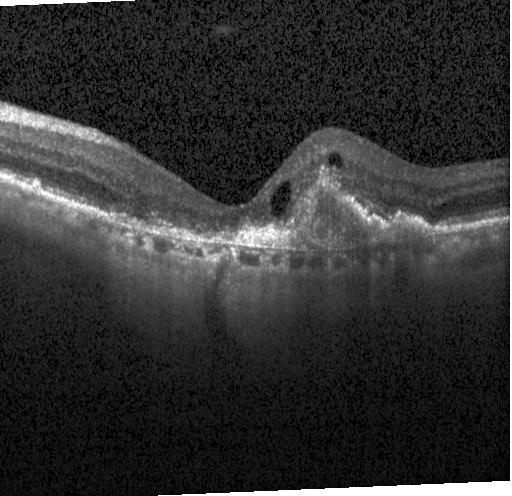 Through the macula · retinal OCT cross-section — Finding: choroidal neovascularization (CNV).